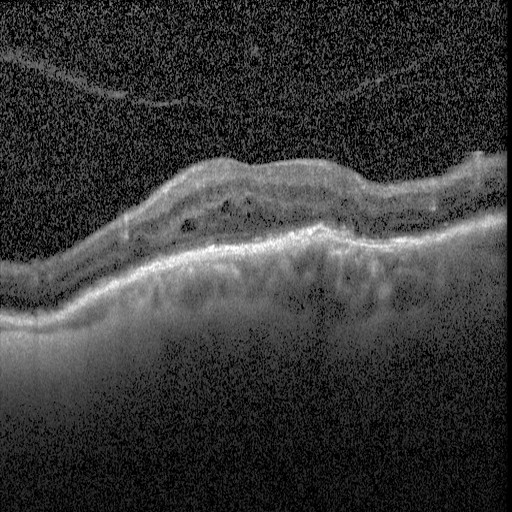
Through the macula. Retinal OCT B-scan.
Diagnosis: diabetic macular edema (DME).